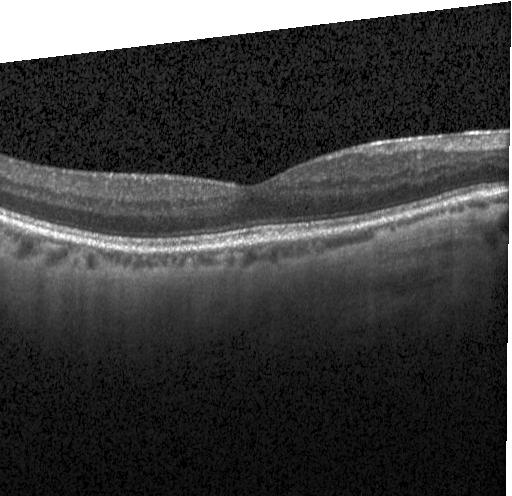
Instrument: Heidelberg Spectralis · retinal OCT cross-section · spectral-domain optical coherence tomography. The scan shows no CNV, no DME, and no drusen.